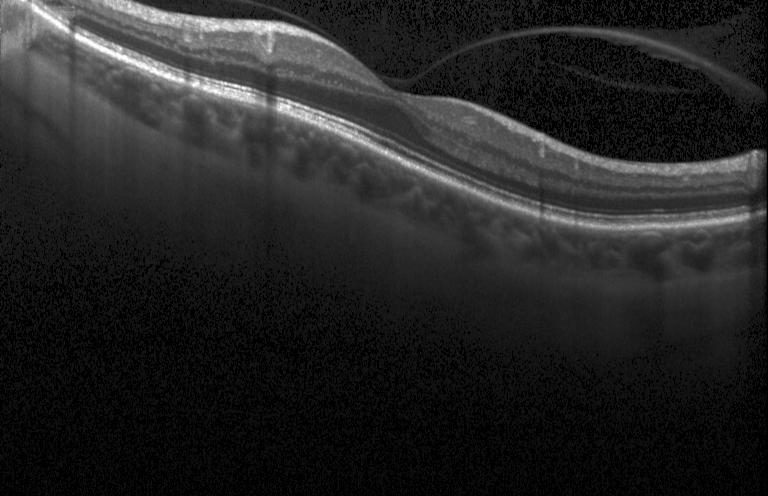
Instrument: Heidelberg Spectralis; retinal OCT cross-section; horizontal scan through the fovea — Impression: no choroidal neovascularization, no diabetic macular edema, and no drusen.